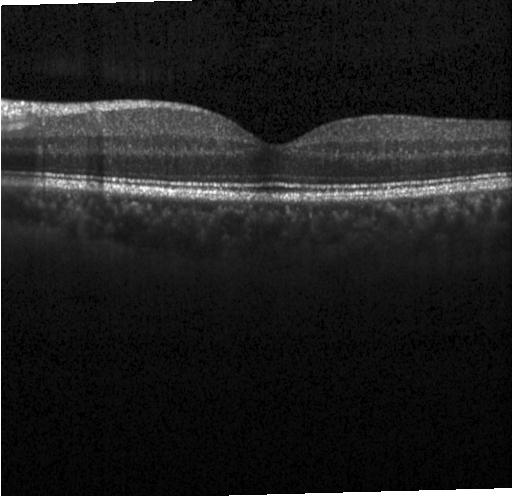 Acquired on a Heidelberg Spectralis. Spectral-domain OCT. OCT line scan. Macular scan — The scan shows no CNV, DME, or drusen.